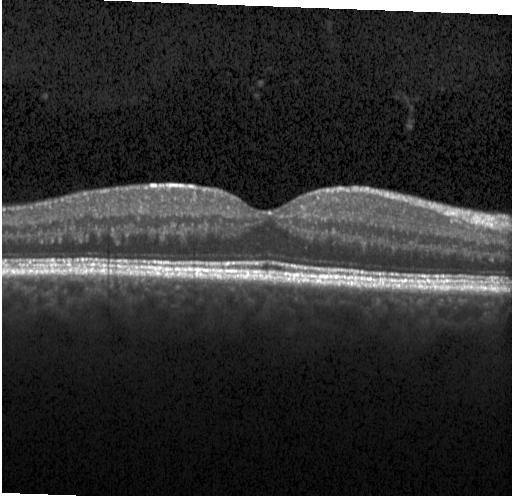 OCT scan showing no CNV, DME, or drusen.